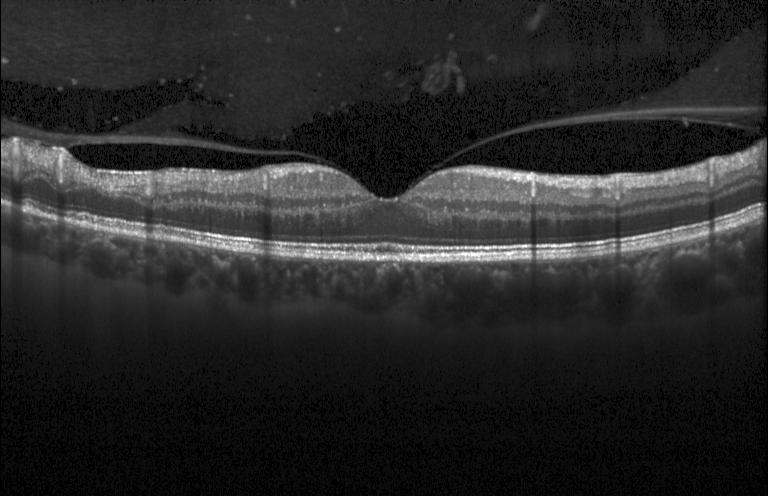

Finding: no evidence of CNV, DME, or drusen.